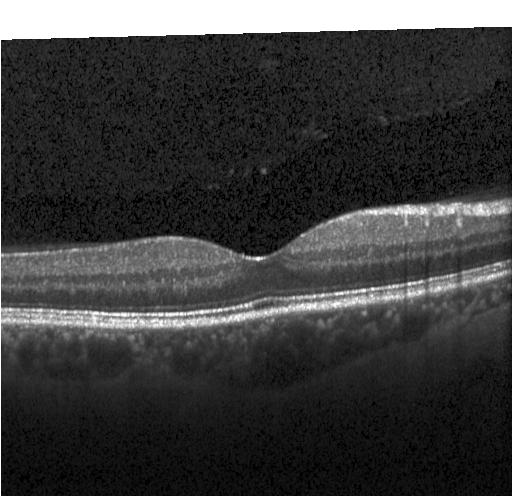

SD-OCT · horizontal scan through the fovea · Heidelberg Spectralis OCT system · optical coherence tomography B-scan. Neither choroidal neovascularization, diabetic macular edema, nor drusen.